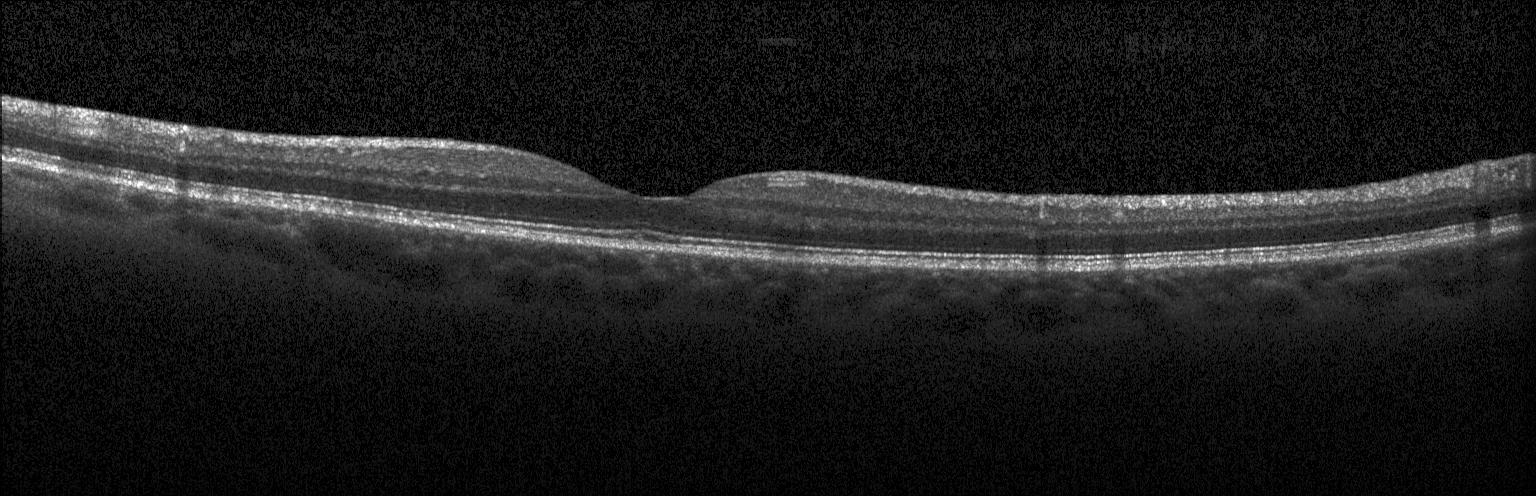

The scan shows neither CNV, DME, nor drusen.